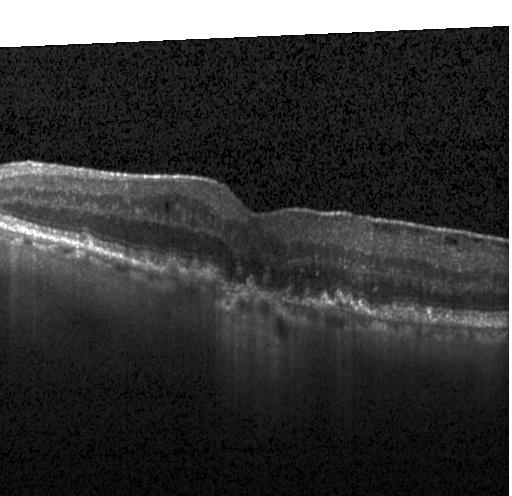 Retinal OCT B-scan.
Assessment: a choroidal neovascular membrane.